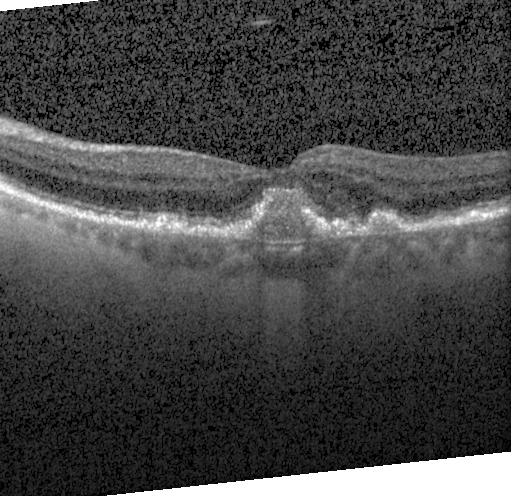
Impression: choroidal neovascularization.